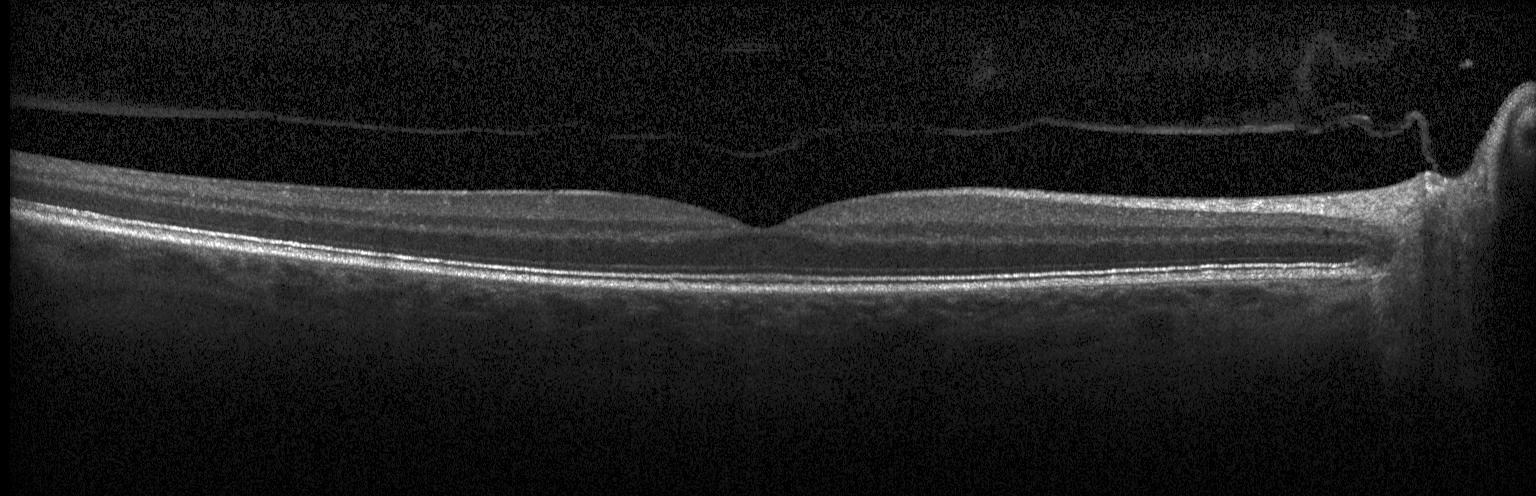
OCT B-scan — Finding: no choroidal neovascularization, no diabetic macular edema, and no drusen.